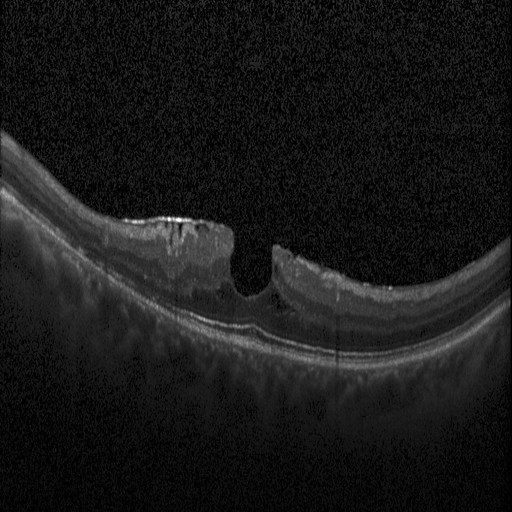
Macular OCT demonstrating DME.